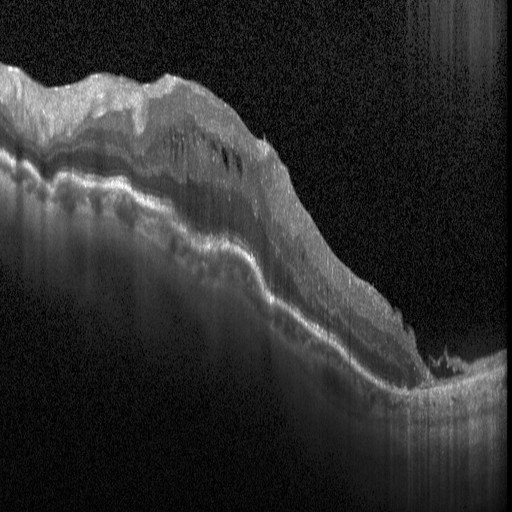
Finding: diabetic macular edema.